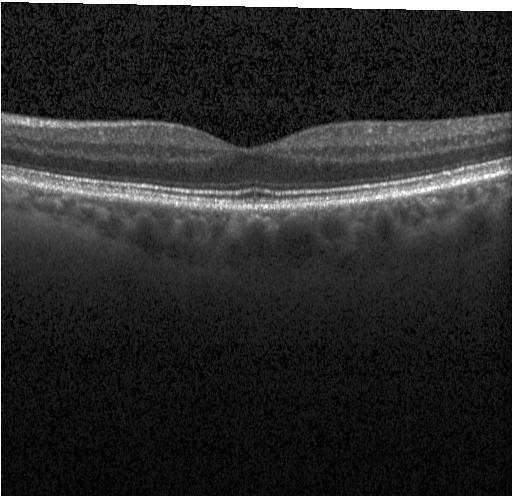 Macular scan · optical coherence tomography B-scan.
Impression: no choroidal neovascularization, diabetic macular edema, or drusen.